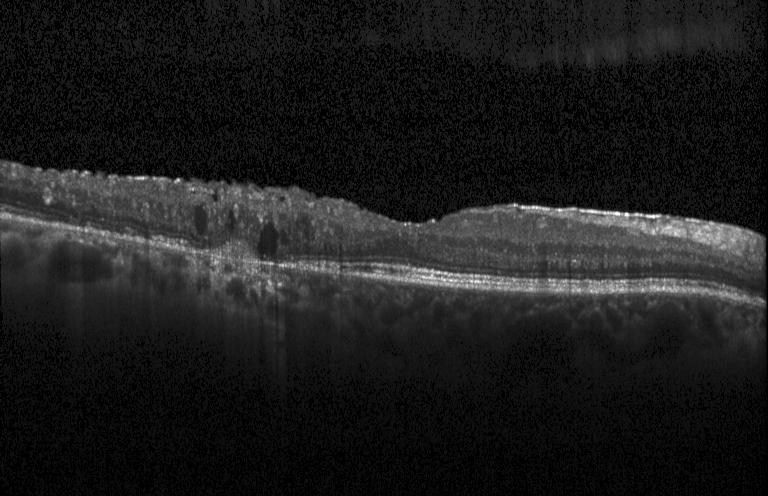 OCT line scan. Instrument: Heidelberg Spectralis. Centered on the fovea — Impression: diabetic macular edema (DME).